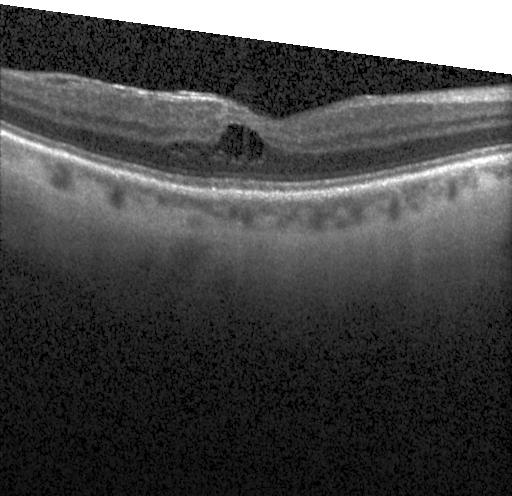 Heidelberg Spectralis. Retinal OCT B-scan. SD-OCT
Assessment: diabetic macular edema.